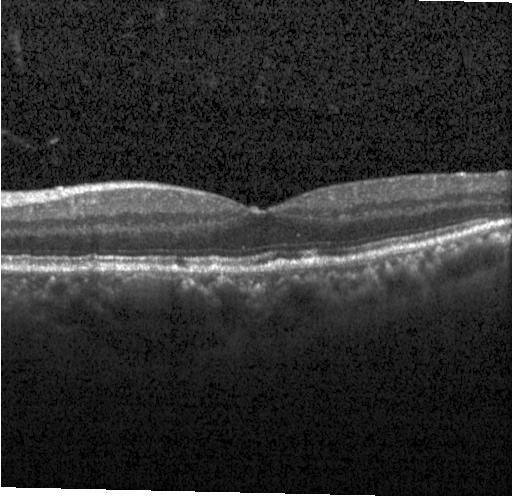
Macular OCT demonstrating multiple drusen.